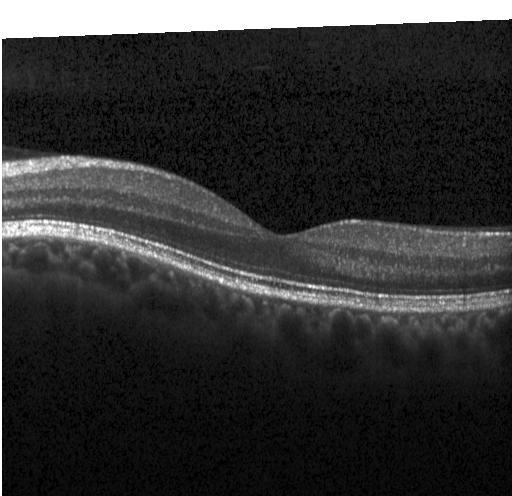

Impression: no choroidal neovascularization, diabetic macular edema, or drusen.